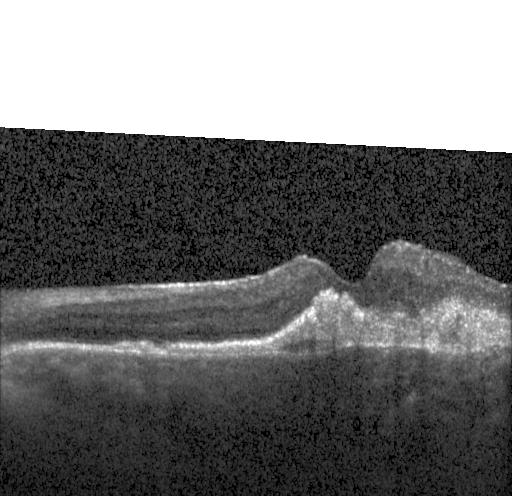 OCT B-scan — Diagnosis: a choroidal neovascular membrane.